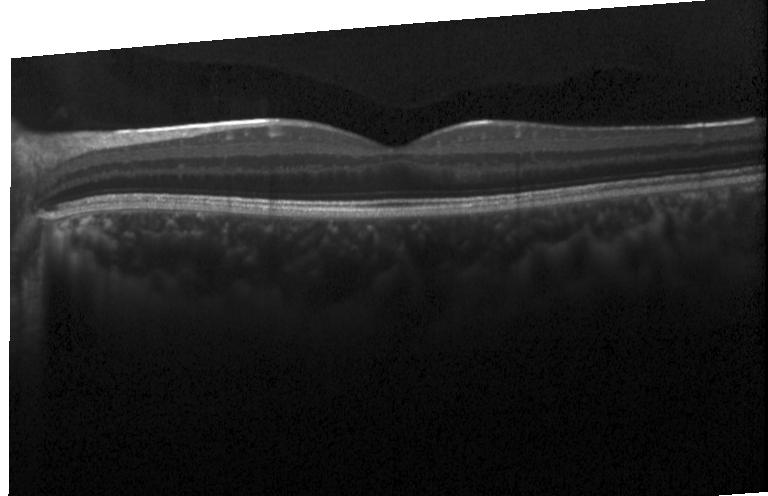

Spectral-domain OCT, instrument: Heidelberg Spectralis, optical coherence tomography B-scan, through the macula
Dx: no CNV, no DME, and no drusen.